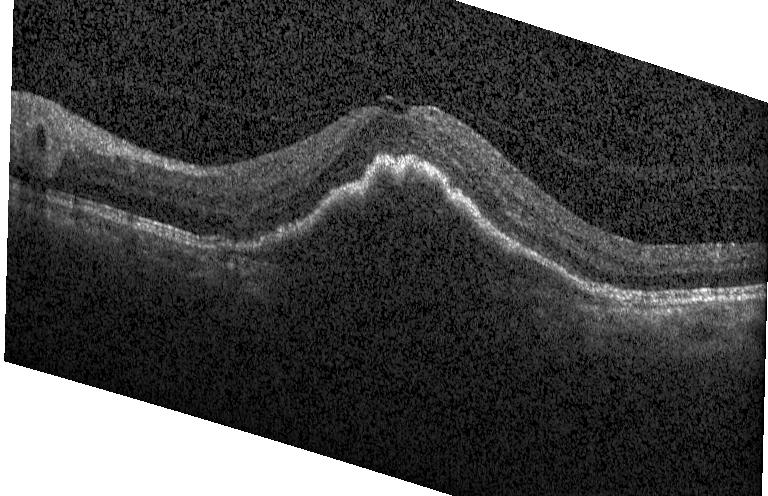 Acquired on a Heidelberg Spectralis; spectral-domain optical coherence tomography; through the macula; optical coherence tomography scan.
Assessment: choroidal neovascularization.